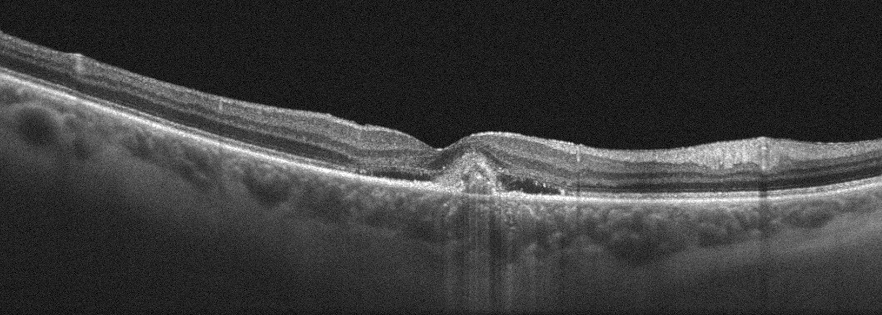 Instrument: Optovue Avanti RTVue XR · OCT line scan. Finding: age-related macular degeneration (AMD).